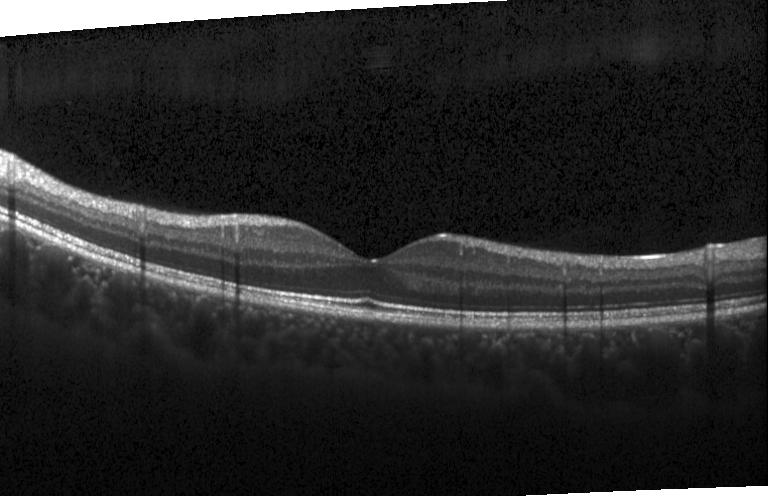 Retinal OCT cross-section, spectral-domain optical coherence tomography, Heidelberg Spectralis OCT system
This B-scan demonstrates no choroidal neovascularization, no diabetic macular edema, and no drusen.